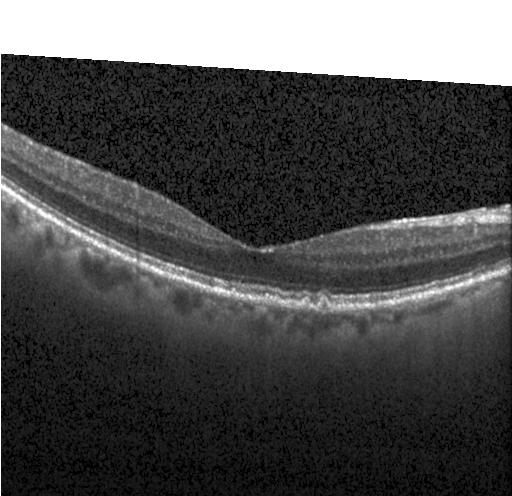

Through the macula. Optical coherence tomography B-scan. Acquired on a Heidelberg Spectralis — Assessment: drusen.